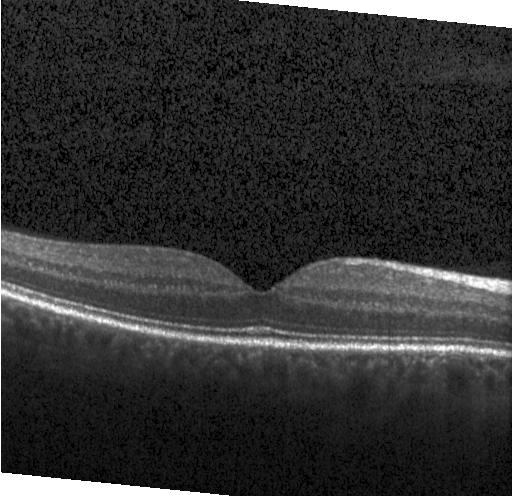

Assessment: neither choroidal neovascularization, diabetic macular edema, nor drusen.